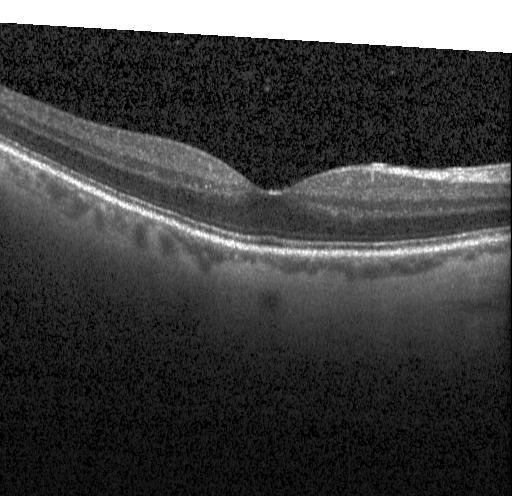 OCT B-scan. Instrument: Heidelberg Spectralis
Neither CNV, DME, nor drusen.